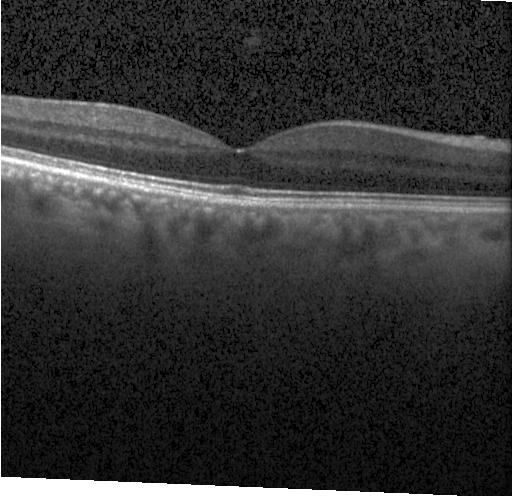 Finding: no choroidal neovascularization, diabetic macular edema, or drusen.